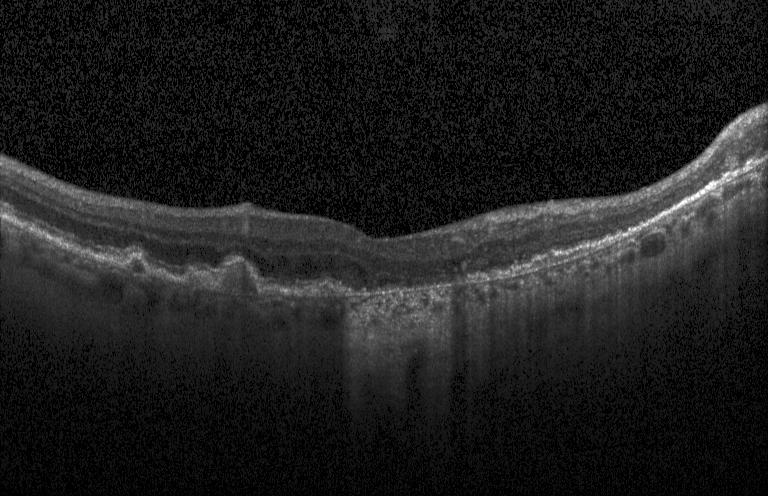
Heidelberg Spectralis; retinal OCT B-scan; spectral-domain optical coherence tomography
The scan shows a choroidal neovascular membrane.